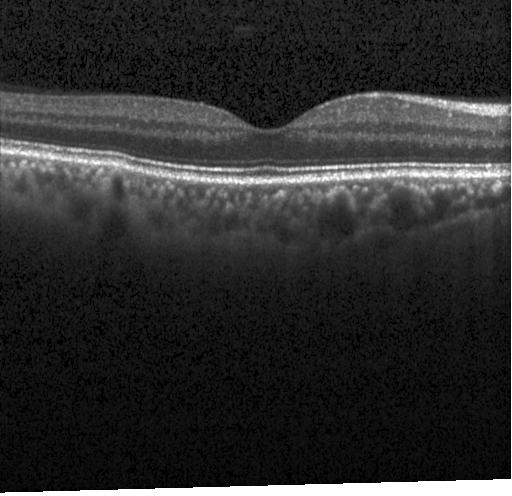
OCT scan showing no evidence of CNV, DME, or drusen.